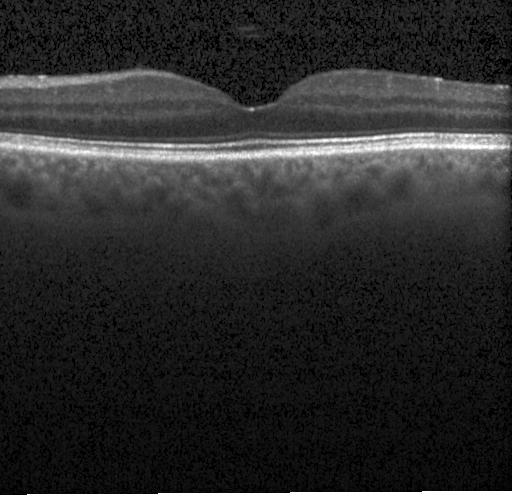 Impression: no CNV, no DME, and no drusen.